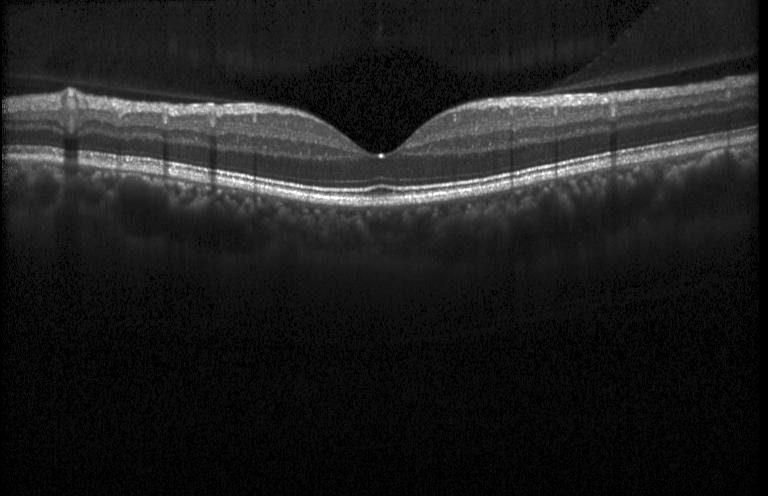
Optical coherence tomography scan. Acquired on a Heidelberg Spectralis. Macular scan.
Diagnosis: no evidence of choroidal neovascularization, diabetic macular edema, or drusen.